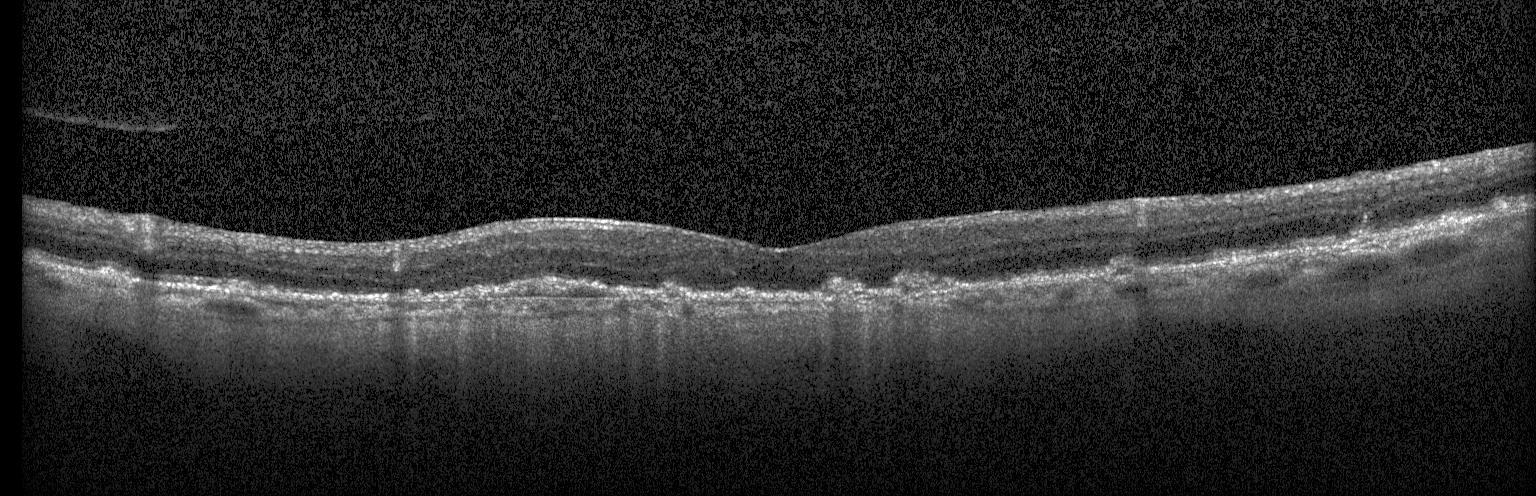
Macular OCT demonstrating a choroidal neovascular membrane.